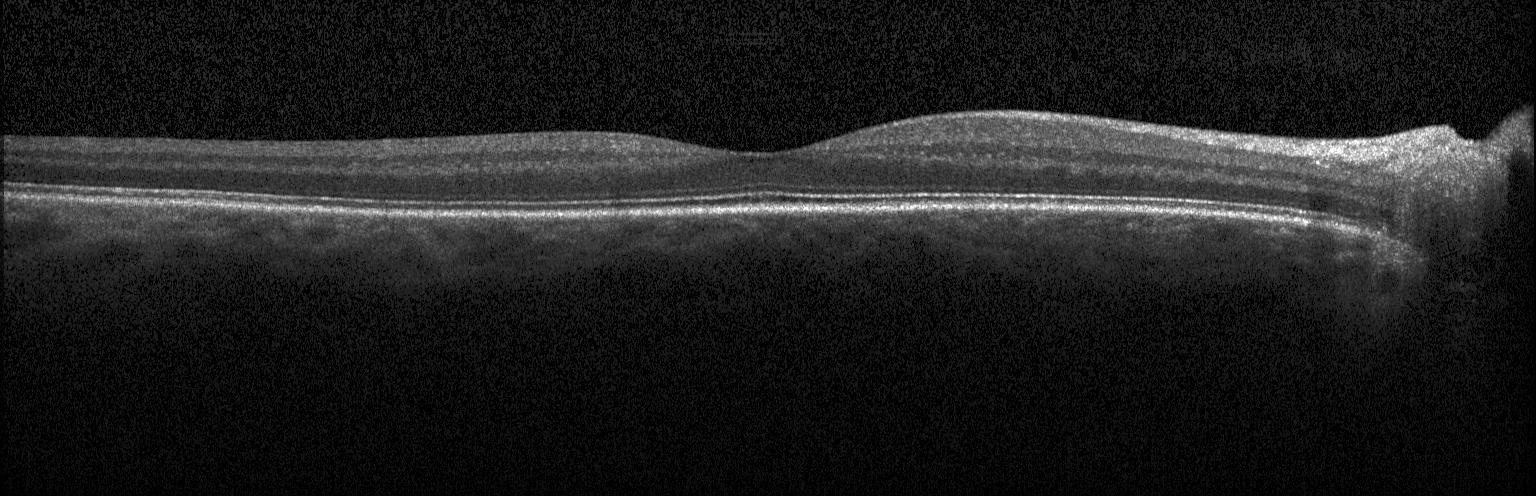 Instrument: Heidelberg Spectralis · retinal OCT B-scan — Impression: no evidence of choroidal neovascularization, diabetic macular edema, or drusen.